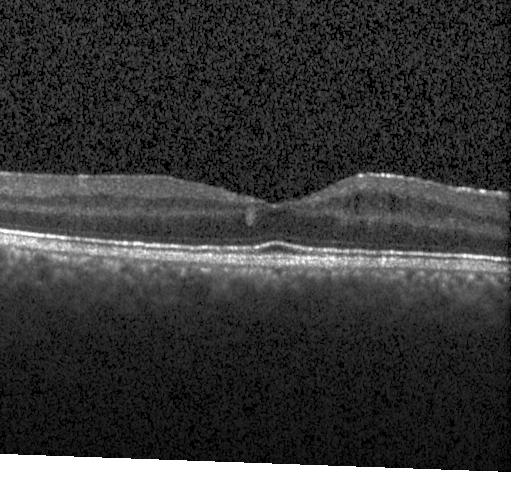

Diagnosis: diabetic macular edema (DME).